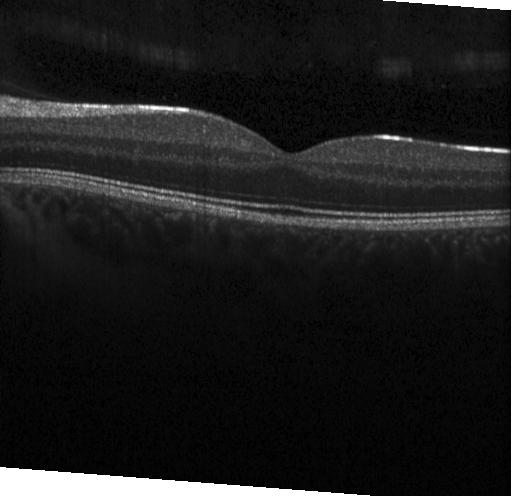 Macular OCT demonstrating neither choroidal neovascularization, diabetic macular edema, nor drusen.